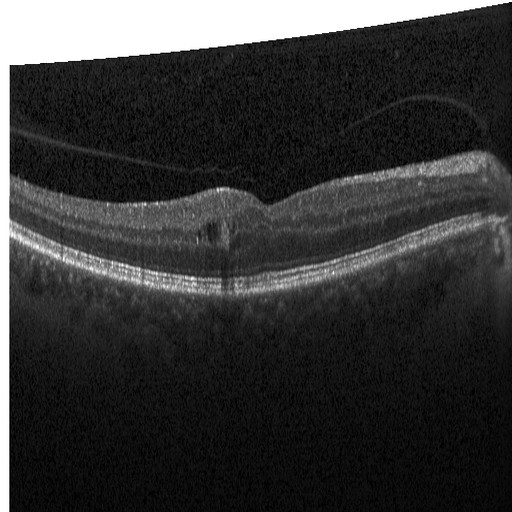 OCT line scan — The scan shows DME.